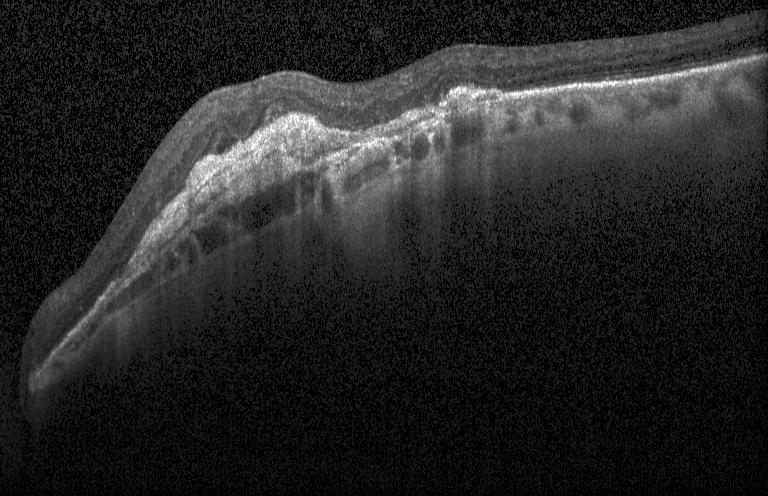 Optical coherence tomography scan — Macular OCT: choroidal neovascularization (CNV).